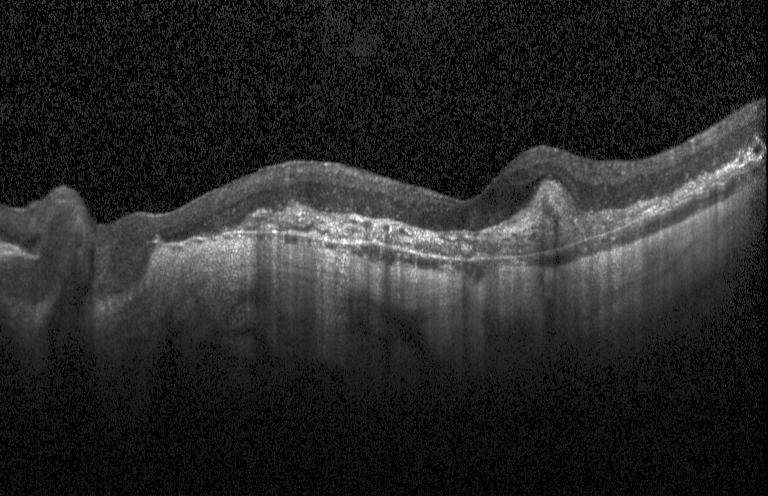
Fovea-centered. OCT B-scan. Spectral-domain optical coherence tomography. Heidelberg Spectralis OCT system — Impression: choroidal neovascularization (CNV).